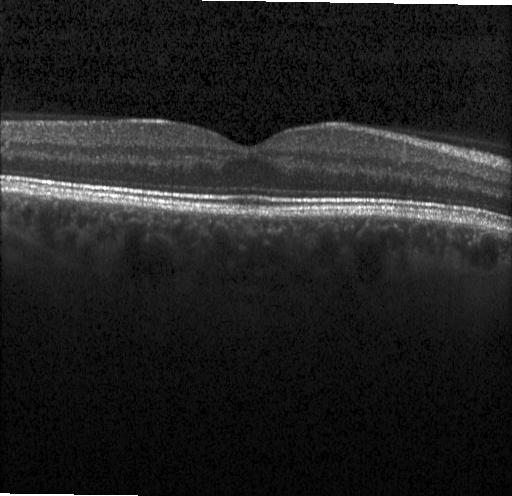 Heidelberg Spectralis OCT system. Spectral-domain optical coherence tomography. Retinal OCT B-scan. Macular OCT: no CNV, no DME, and no drusen.